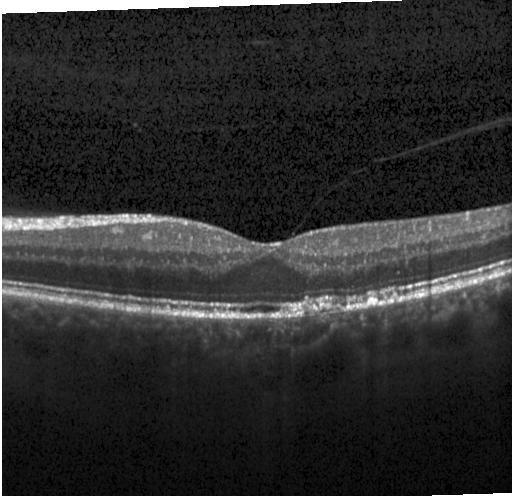
Impression: drusen.